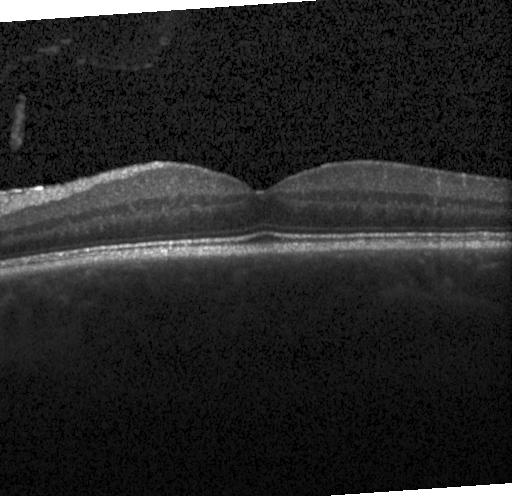
Diagnosis: neither CNV, DME, nor drusen.